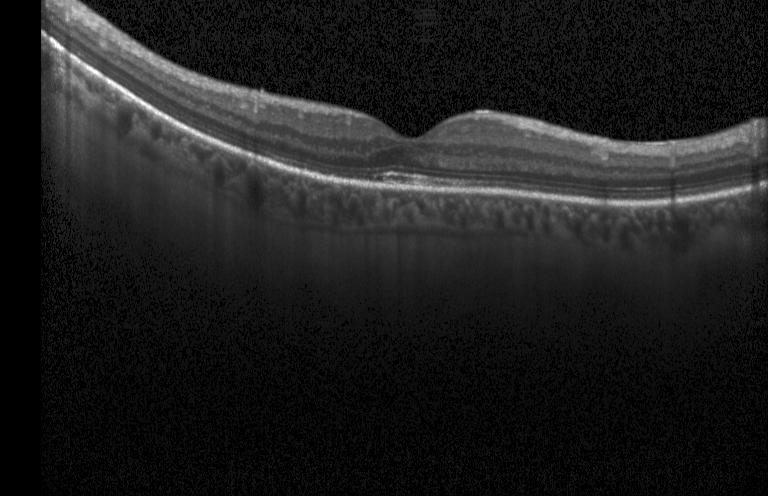 Finding: no CNV, no DME, and no drusen.